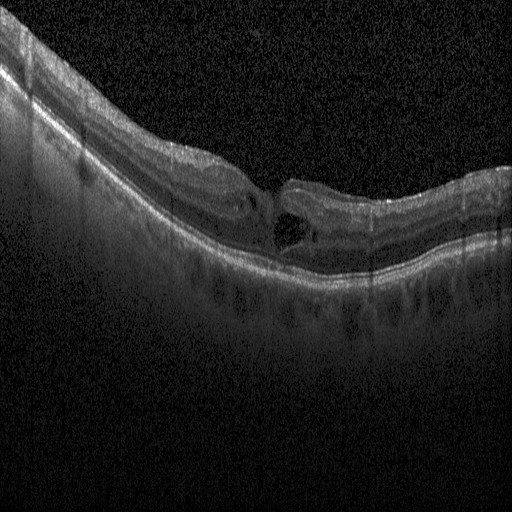
SD-OCT · optical coherence tomography scan — Assessment: diabetic macular edema (DME).